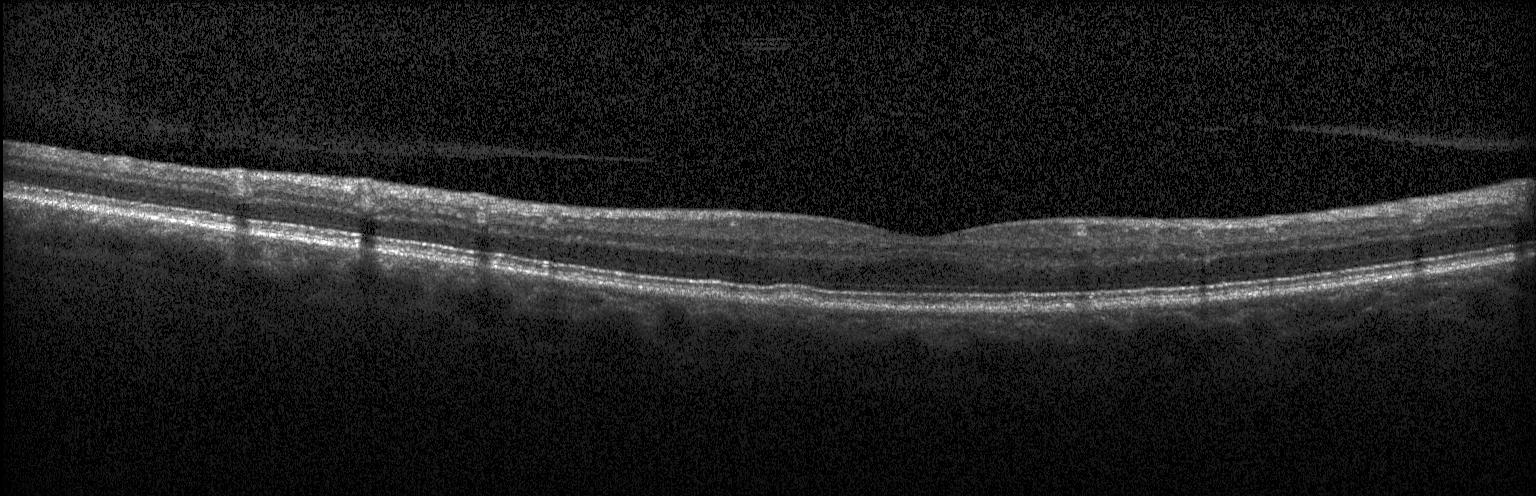 Heidelberg Spectralis. Spectral-domain optical coherence tomography. Through the macula. Optical coherence tomography B-scan. This B-scan demonstrates no choroidal neovascularization, diabetic macular edema, or drusen.